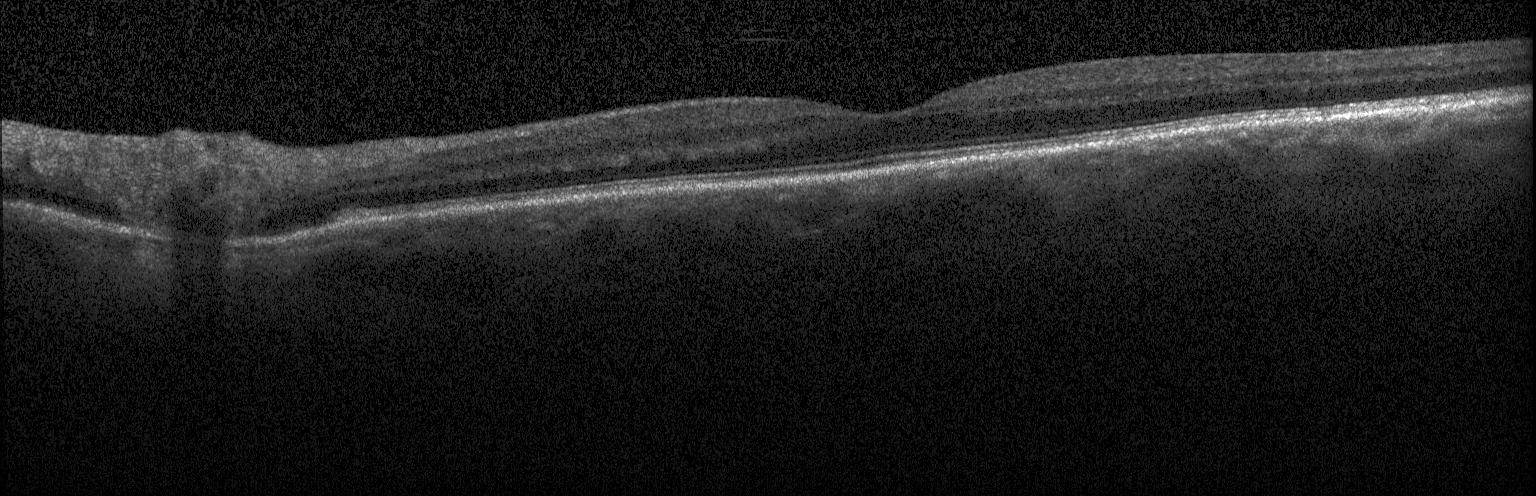

The scan shows no choroidal neovascularization, diabetic macular edema, or drusen.